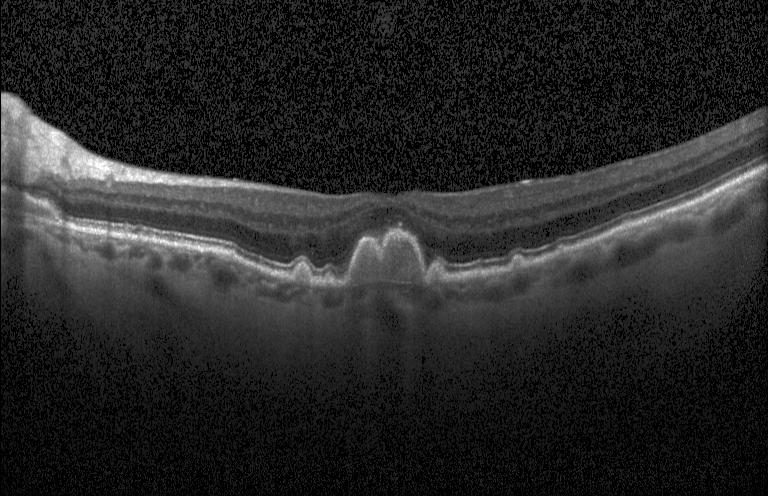

Macular OCT: multiple drusen.